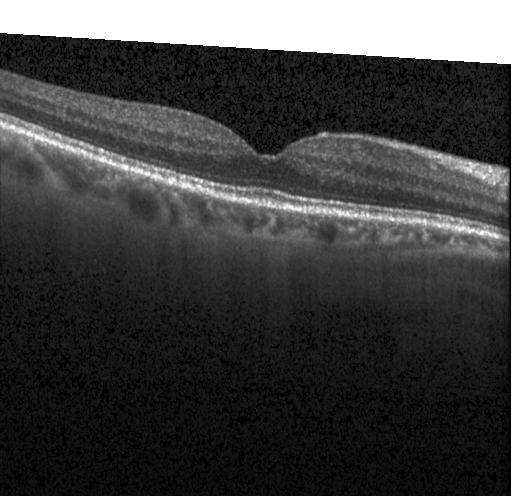 Macular OCT: no choroidal neovascularization, diabetic macular edema, or drusen.